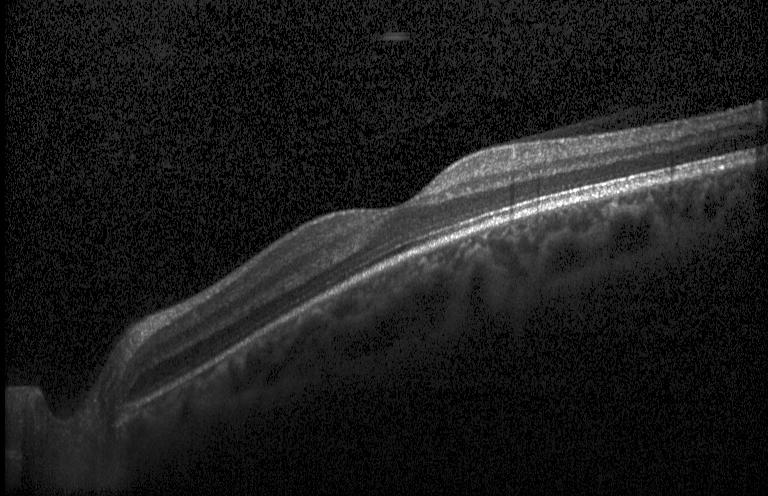 OCT B-scan
Dx: neither choroidal neovascularization, diabetic macular edema, nor drusen.